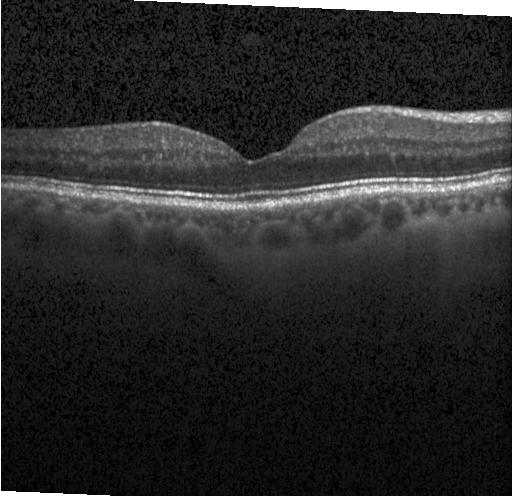 OCT B-scan showing no evidence of choroidal neovascularization, diabetic macular edema, or drusen.